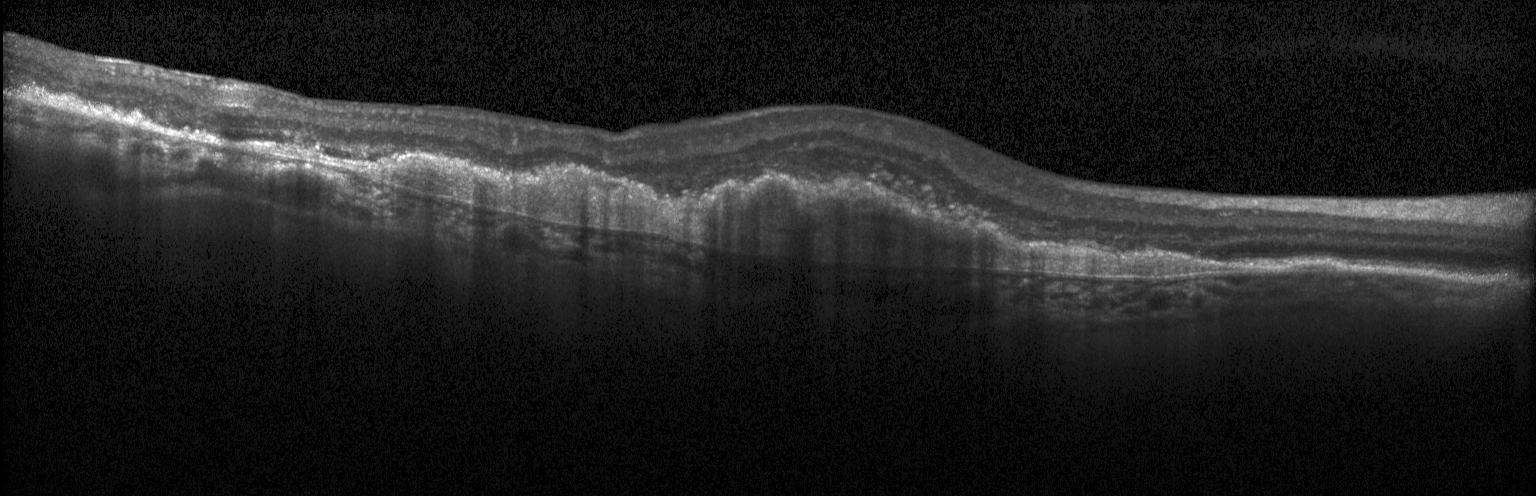
Acquired on a Heidelberg Spectralis, optical coherence tomography B-scan, fovea-centered, spectral-domain optical coherence tomography.
OCT finding: CNV.